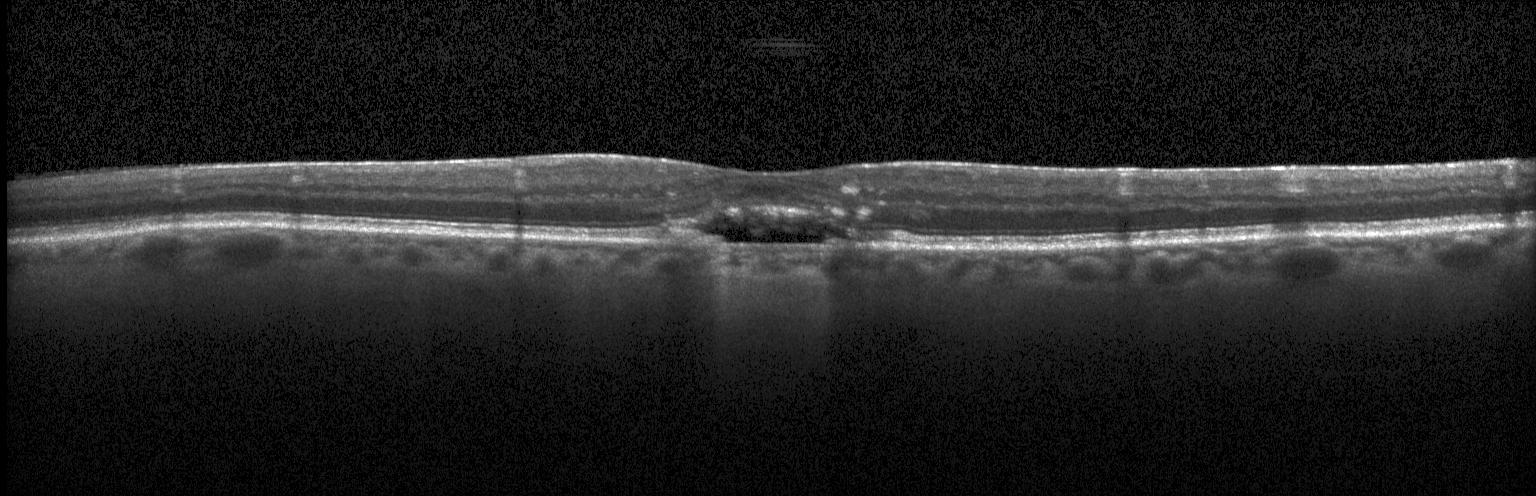
OCT scan showing a choroidal neovascular membrane.